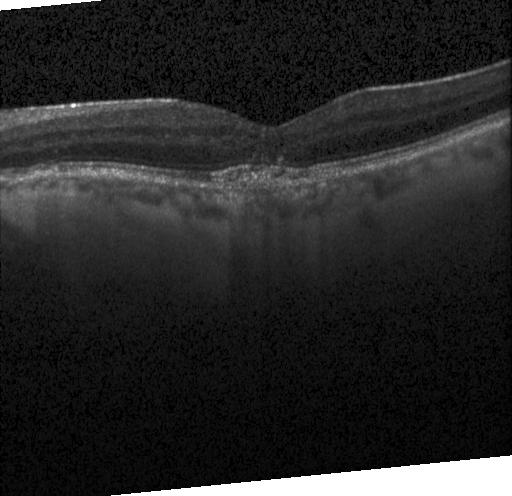 OCT B-scan — The scan shows a choroidal neovascular membrane.